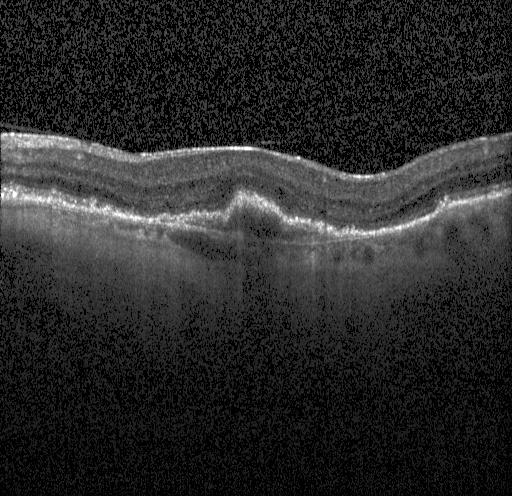
Assessment: a choroidal neovascular membrane.